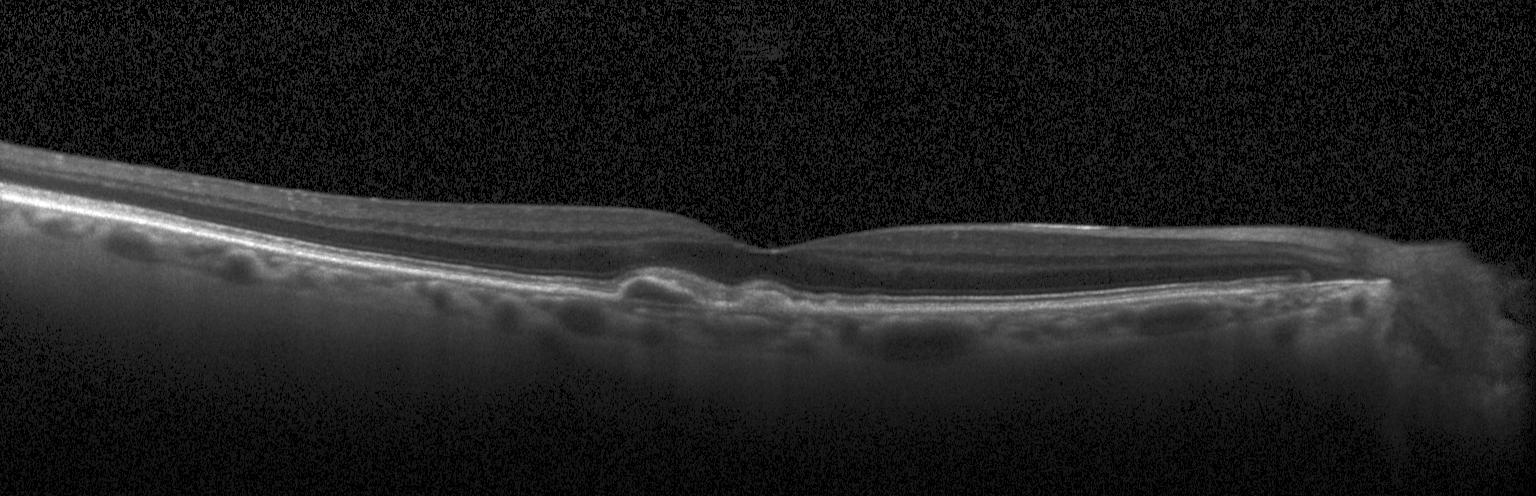

Instrument: Heidelberg Spectralis, fovea-centered, retinal OCT cross-section. This B-scan demonstrates a choroidal neovascular membrane.